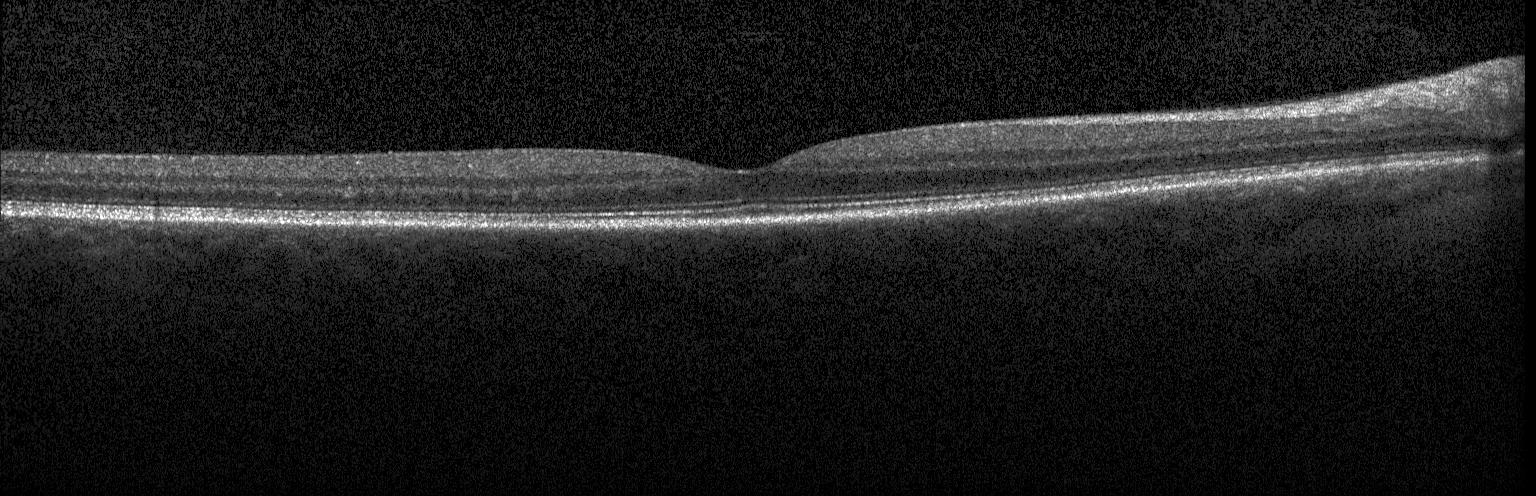

Macular OCT: no evidence of choroidal neovascularization, diabetic macular edema, or drusen.